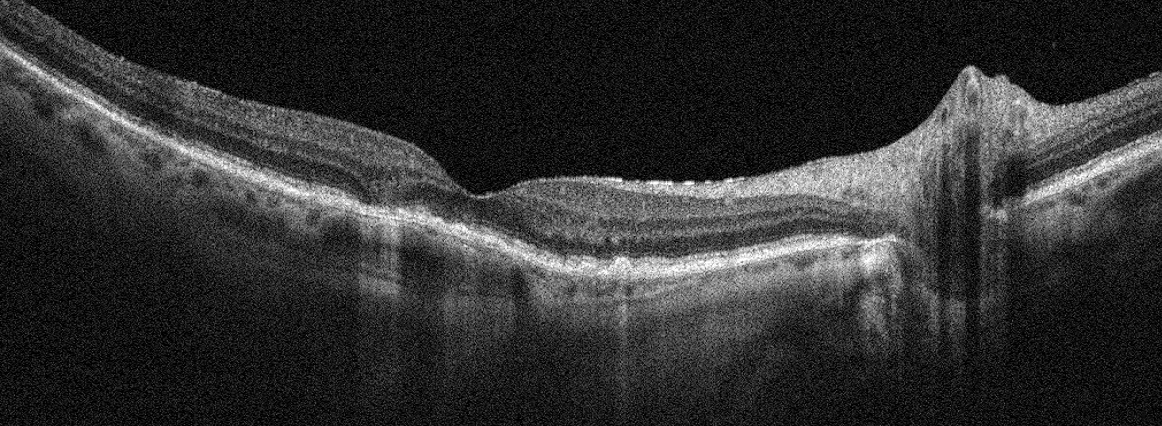
Oculus dexter; optical coherence tomography B-scan. Finding: AMD.